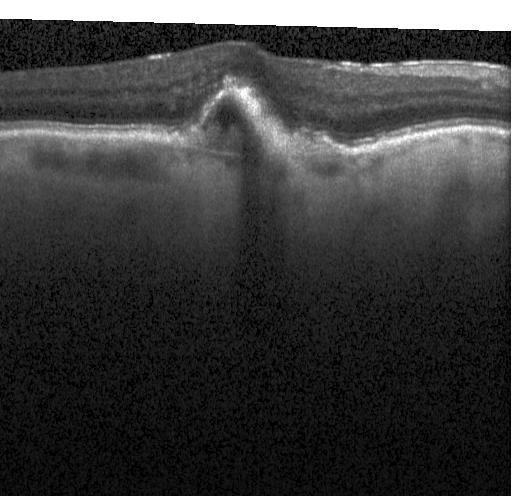

A choroidal neovascular membrane.